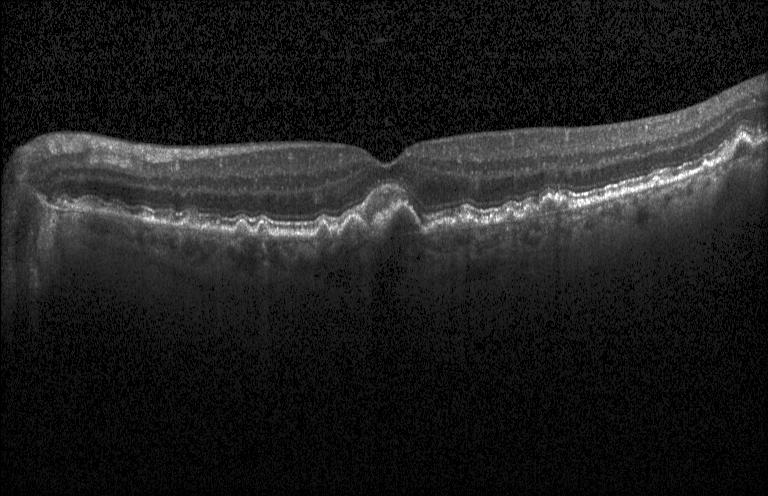 Retinal OCT B-scan; SD-OCT; Heidelberg Spectralis OCT system.
Finding: choroidal neovascularization (CNV).